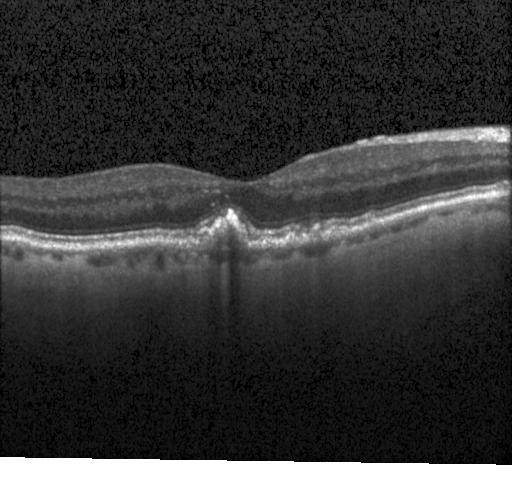

OCT B-scan showing sub-RPE drusenoid deposits.